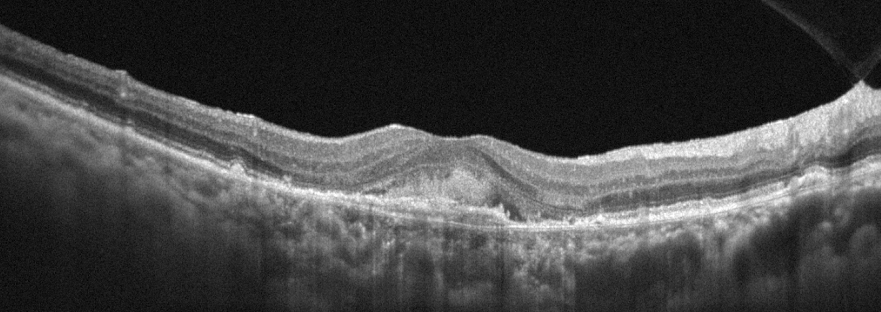
Retinal OCT B-scan, macular scan. Assessment: age-related macular degeneration.